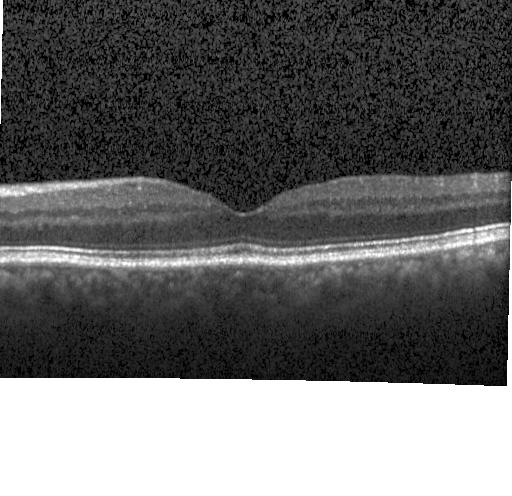
Dx: neither CNV, DME, nor drusen.